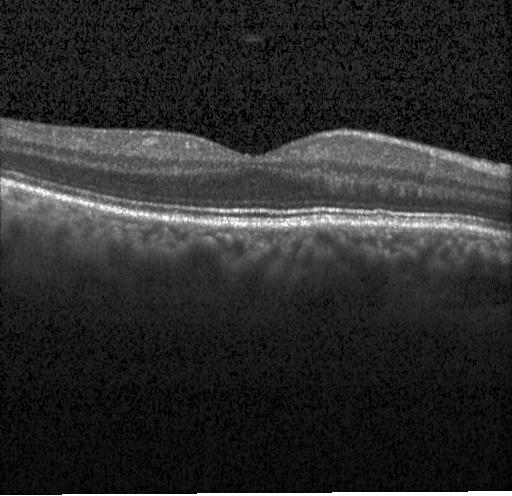
OCT finding: neither CNV, DME, nor drusen.